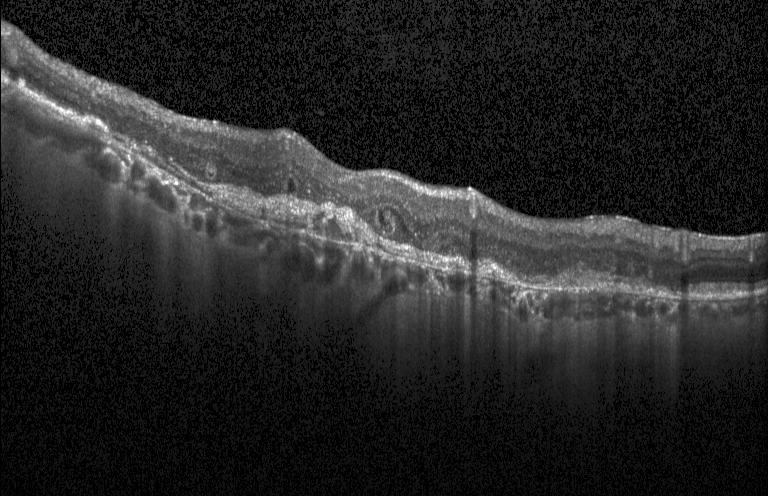

Retinal OCT cross-section — A choroidal neovascular membrane.